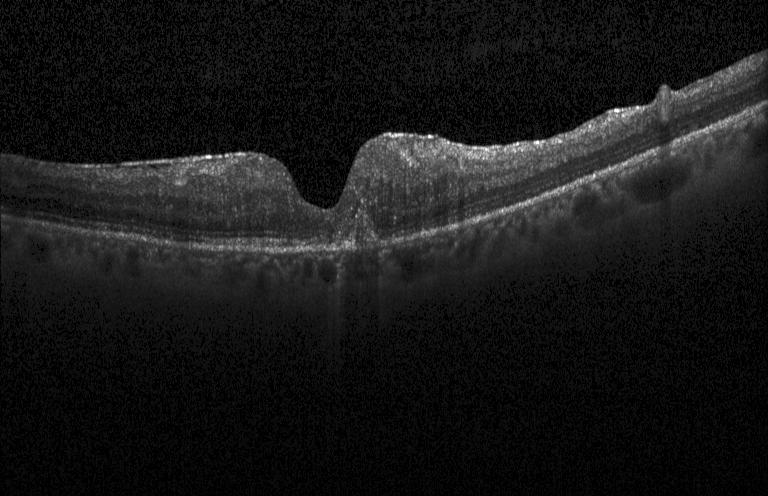

Optical coherence tomography B-scan · acquired on a Heidelberg Spectralis · SD-OCT
Dx: choroidal neovascularization.